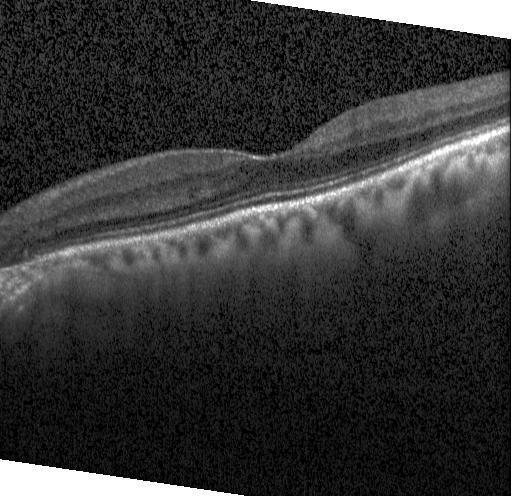
Dx: no evidence of CNV, DME, or drusen.